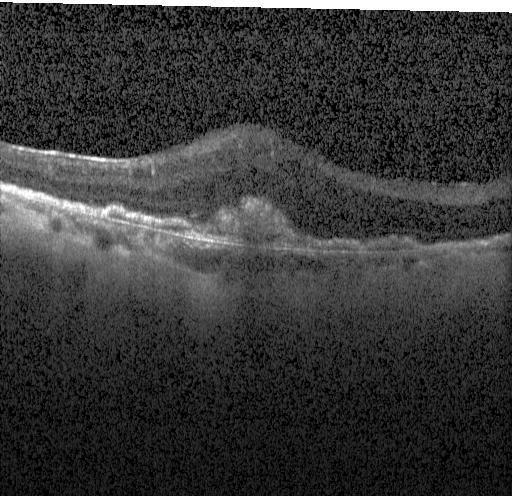
Fovea-centered, OCT B-scan, acquired on a Heidelberg Spectralis. This B-scan demonstrates a choroidal neovascular membrane.